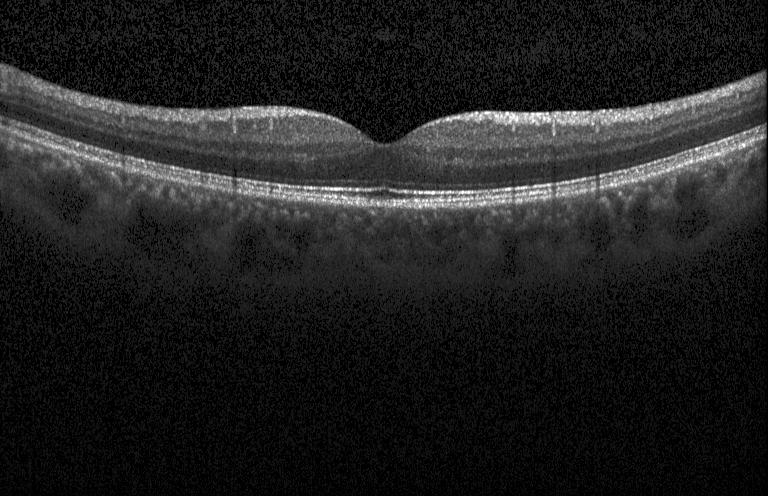

OCT scan showing no evidence of CNV, DME, or drusen.